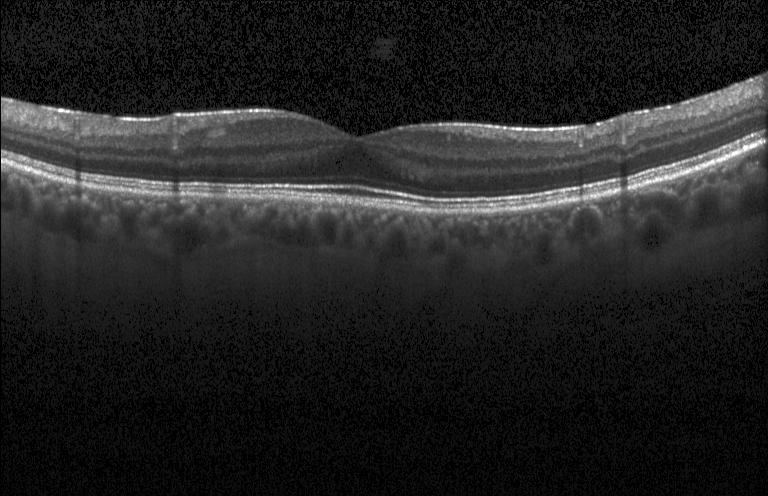

Optical coherence tomography B-scan — Macular OCT: no CNV, DME, or drusen.